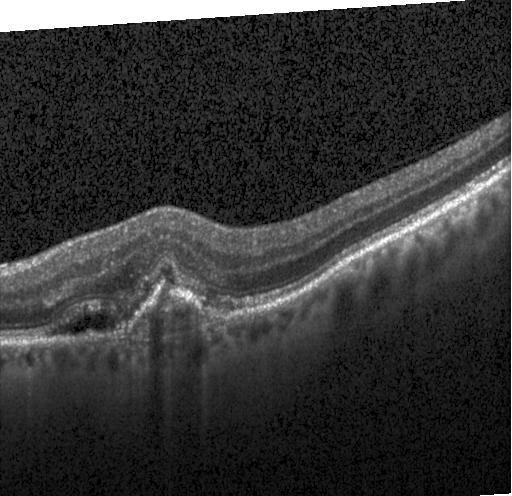

Dx: choroidal neovascularization (CNV).